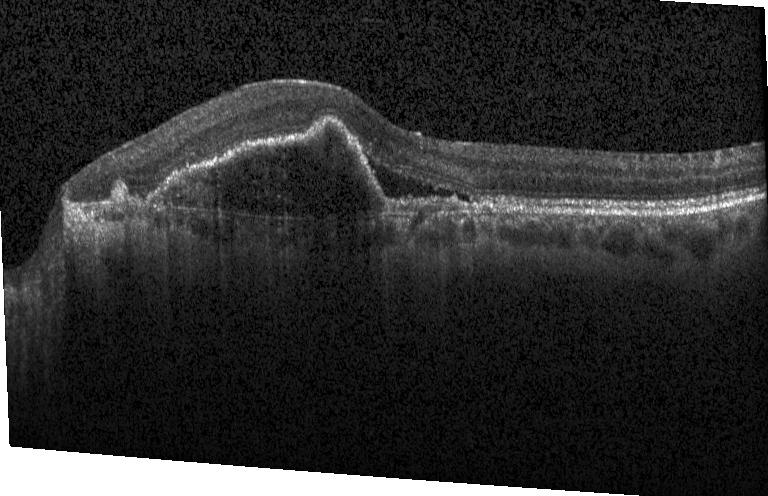
Retinal OCT B-scan
The scan shows a choroidal neovascular membrane.